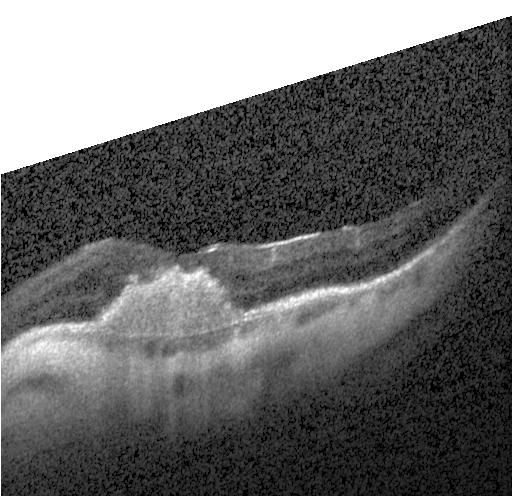
Optical coherence tomography B-scan
This B-scan demonstrates a choroidal neovascular membrane.